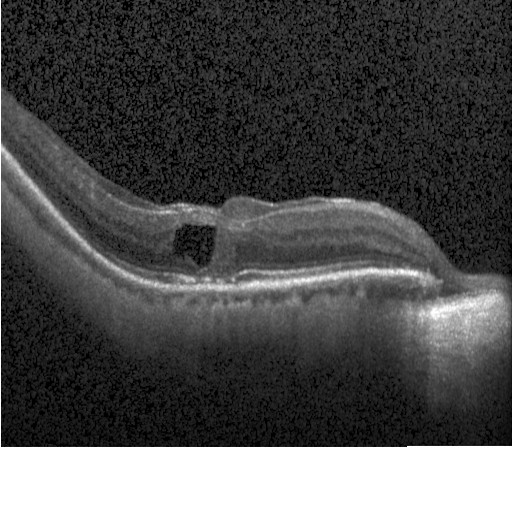 Optical coherence tomography B-scan; through the macula; spectral-domain optical coherence tomography. Finding: DME.